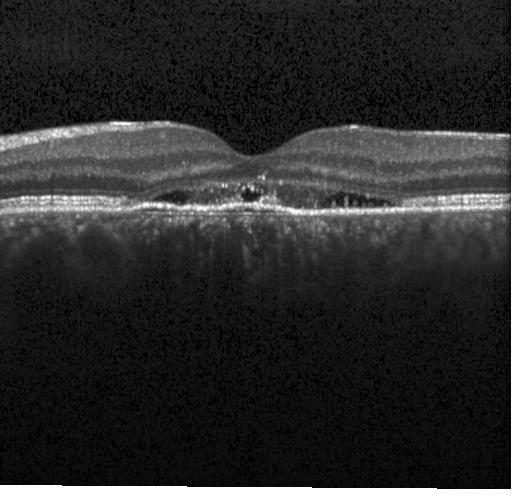
Heidelberg Spectralis. SD-OCT. Optical coherence tomography scan.
Macular OCT: choroidal neovascularization.